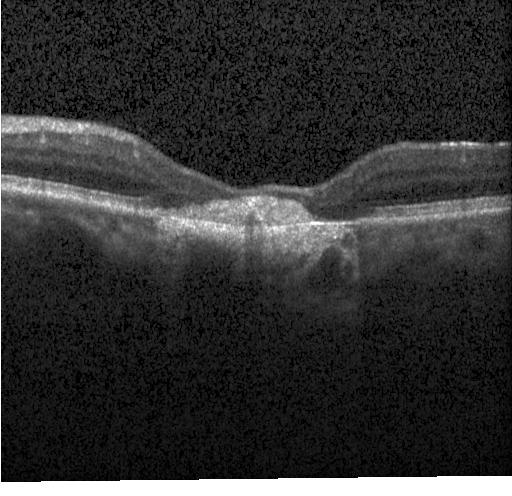
The scan shows choroidal neovascularization.